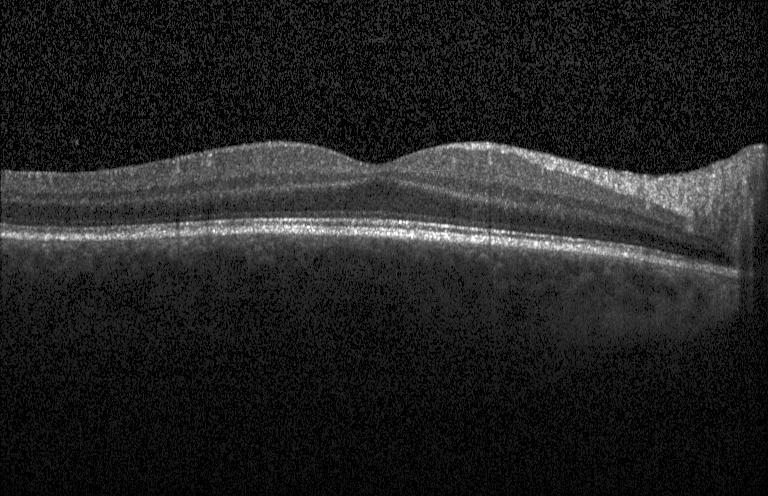

Dx: neither choroidal neovascularization, diabetic macular edema, nor drusen.